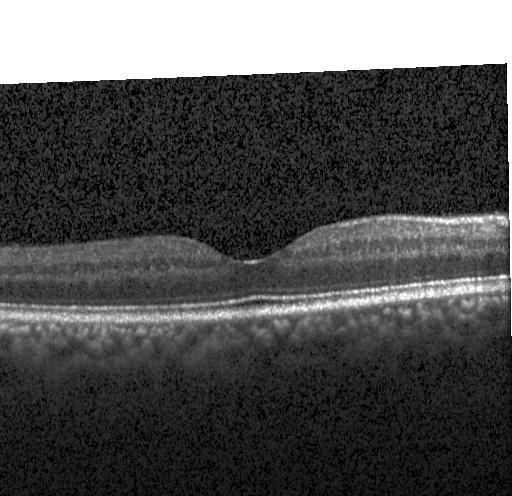

Impression: no choroidal neovascularization, no diabetic macular edema, and no drusen.